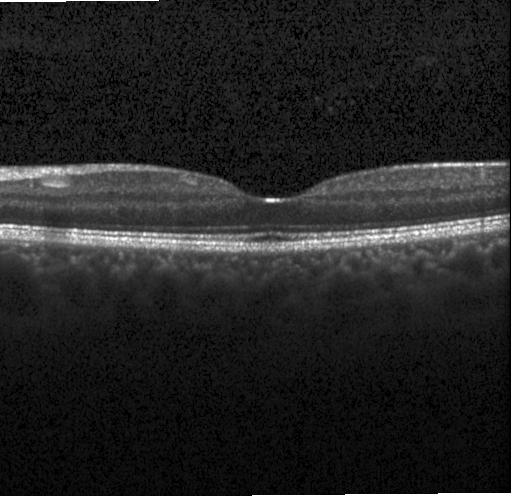 Retinal OCT cross-section
Assessment: no choroidal neovascularization, no diabetic macular edema, and no drusen.